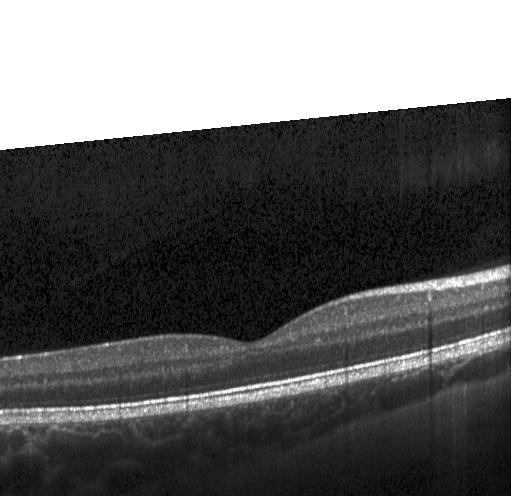 Optical coherence tomography scan; SD-OCT; instrument: Heidelberg Spectralis; through the macula. Impression: neither choroidal neovascularization, diabetic macular edema, nor drusen.